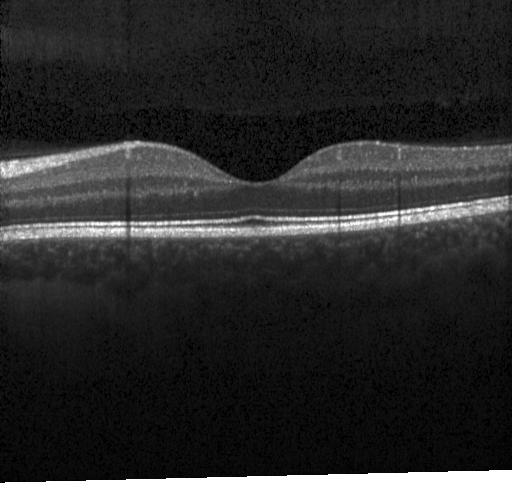 Retinal OCT B-scan. The scan shows no choroidal neovascularization, diabetic macular edema, or drusen.